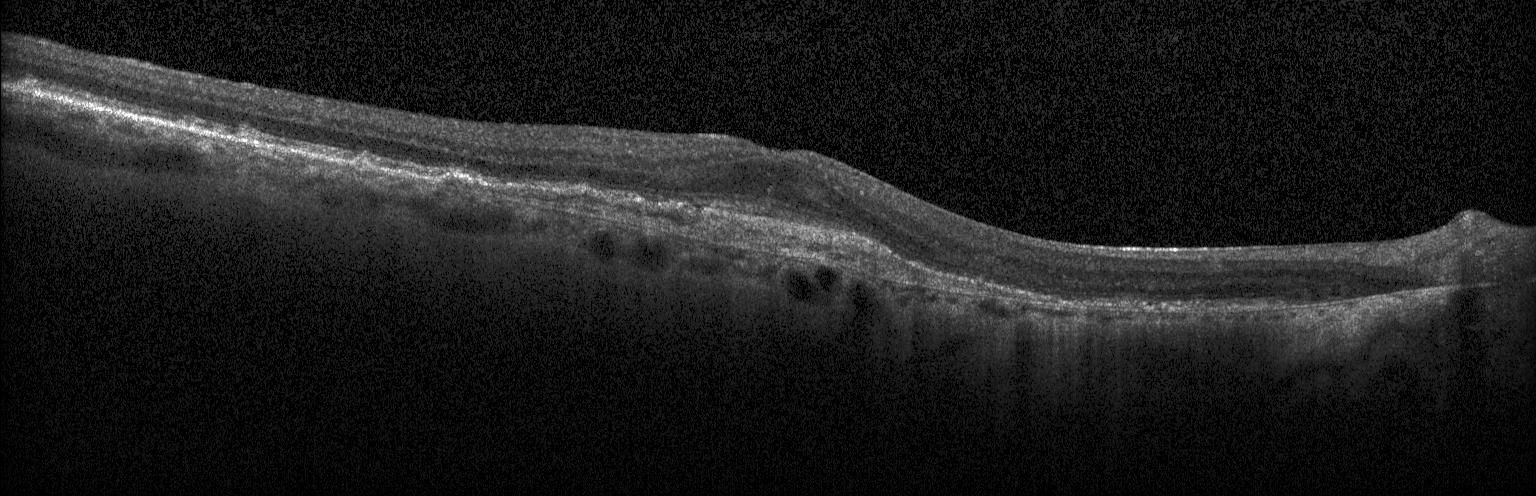

Retinal OCT B-scan.
Macular OCT: choroidal neovascularization.